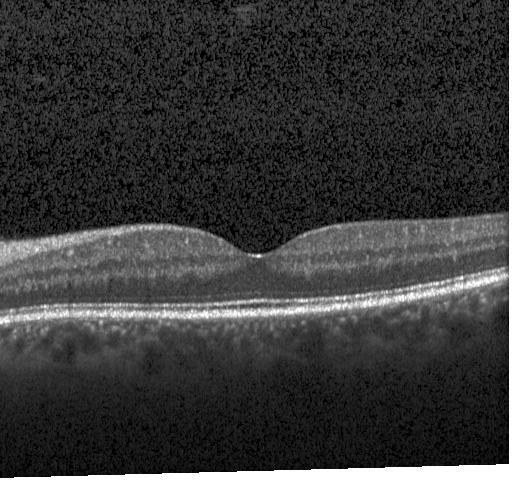
Neither choroidal neovascularization, diabetic macular edema, nor drusen.